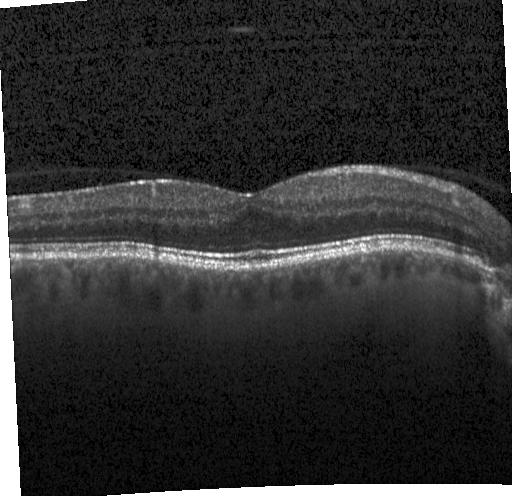 Optical coherence tomography B-scan
OCT finding: neither CNV, DME, nor drusen.